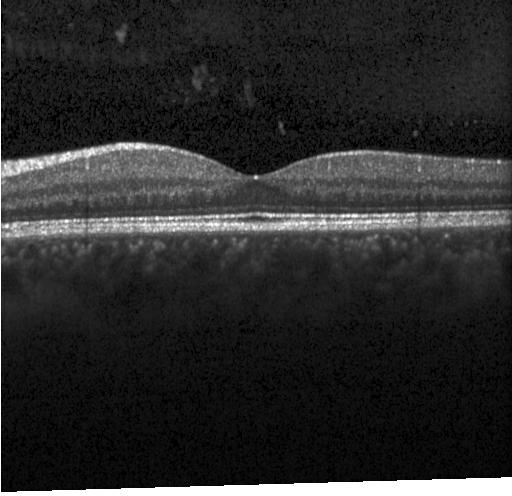 OCT line scan · instrument: Heidelberg Spectralis — Macular OCT: no choroidal neovascularization, diabetic macular edema, or drusen.